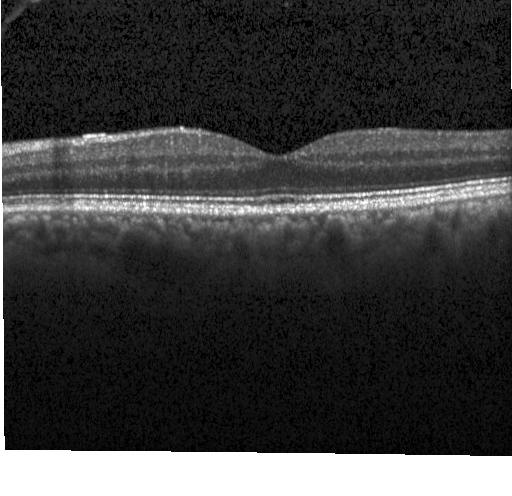

Centered on the fovea · spectral-domain optical coherence tomography · OCT line scan · Heidelberg Spectralis OCT system
Finding: neither choroidal neovascularization, diabetic macular edema, nor drusen.